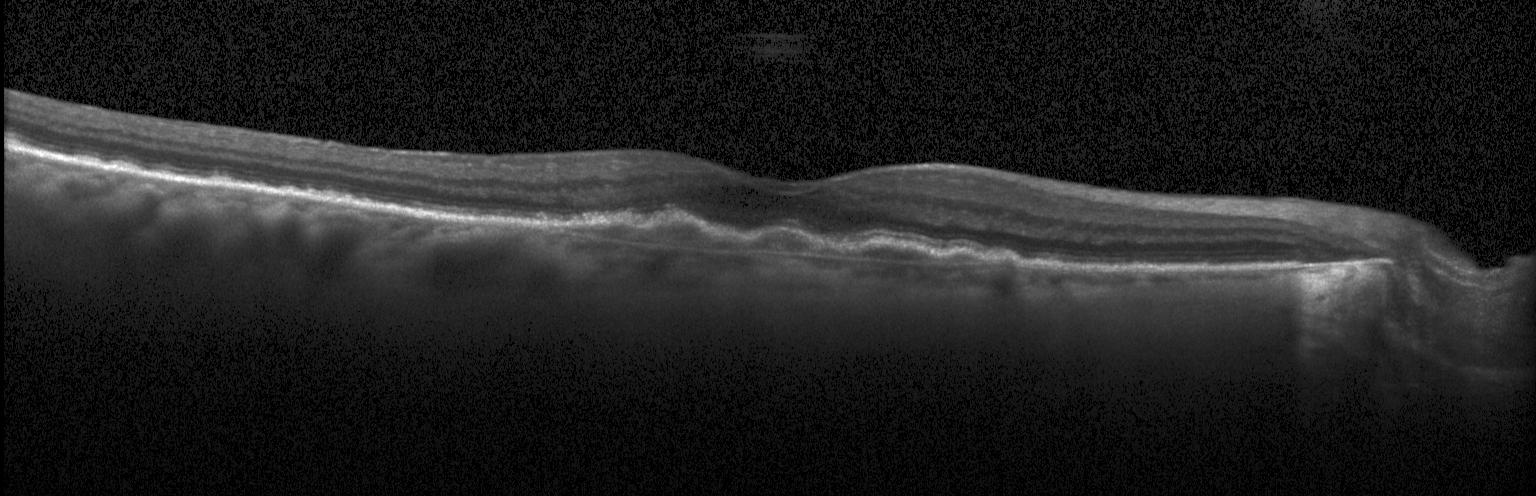

Retinal OCT cross-section showing a choroidal neovascular membrane.